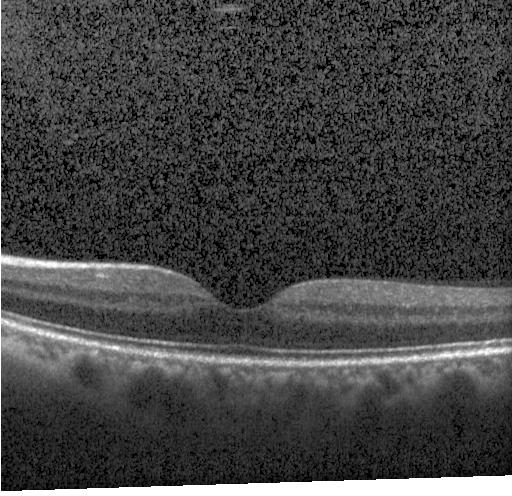 Optical coherence tomography scan; through the macula; instrument: Heidelberg Spectralis; spectral-domain optical coherence tomography
Finding: no evidence of CNV, DME, or drusen.